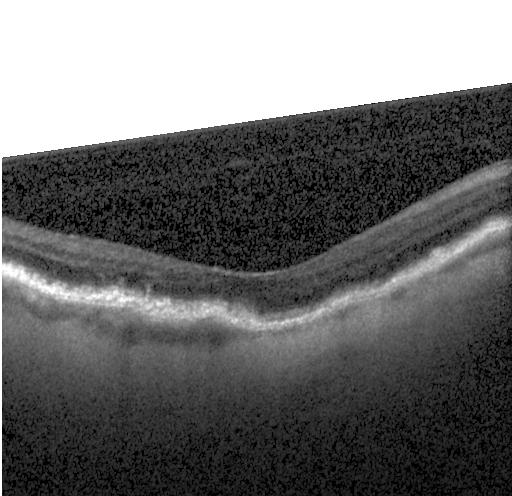

Macular OCT demonstrating a choroidal neovascular membrane.